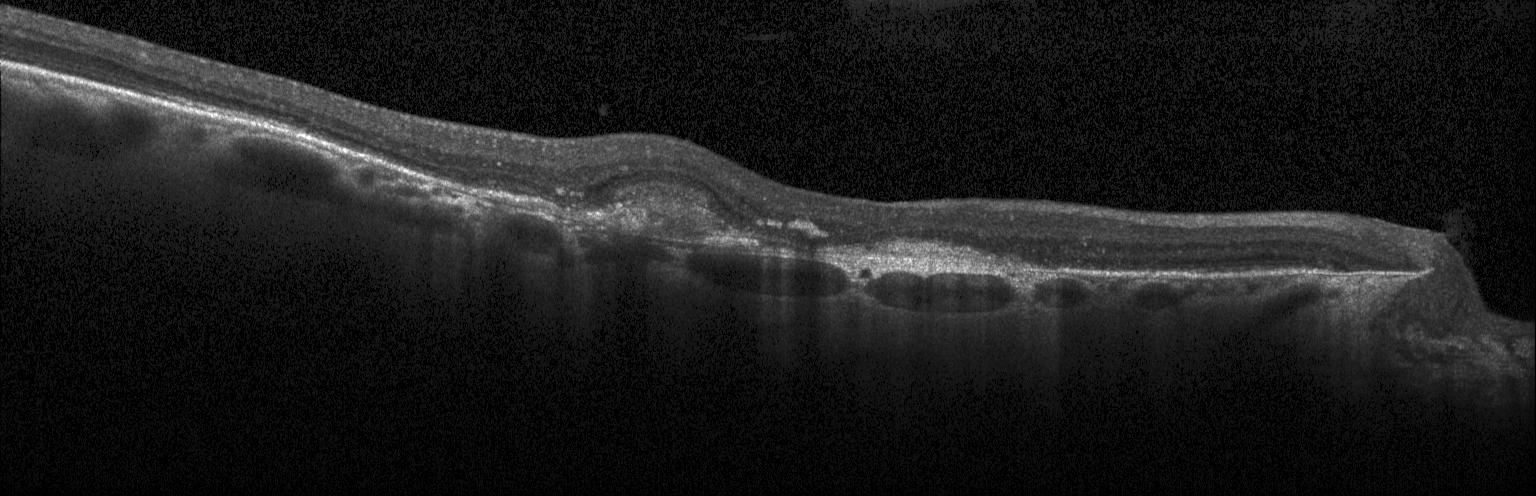

Diagnosis: a choroidal neovascular membrane.